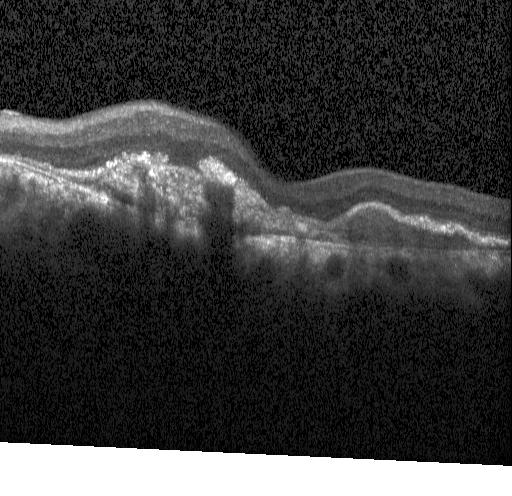
A choroidal neovascular membrane.